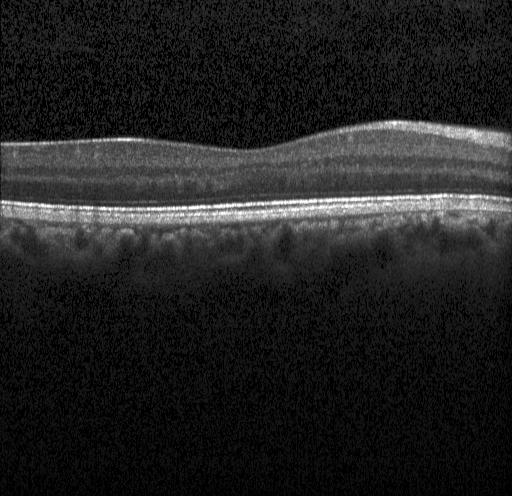 Optical coherence tomography scan. Spectral-domain OCT. Horizontal scan through the fovea.
Impression: no CNV, no DME, and no drusen.